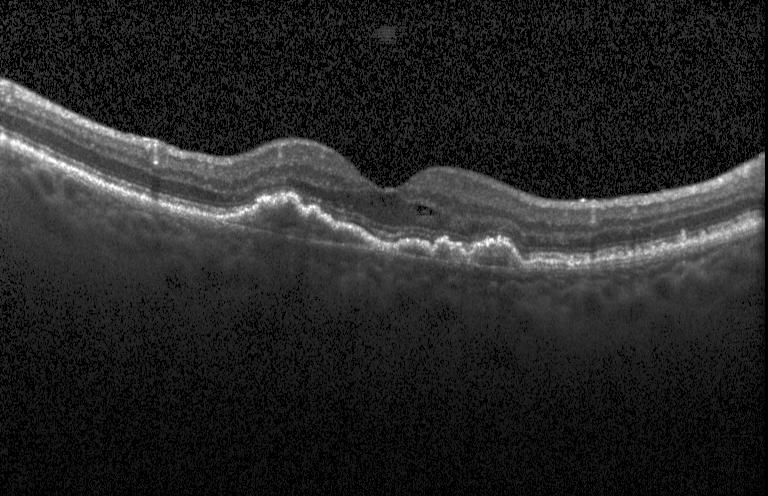
Heidelberg Spectralis OCT system · OCT B-scan · spectral-domain optical coherence tomography. Impression: choroidal neovascularization (CNV).